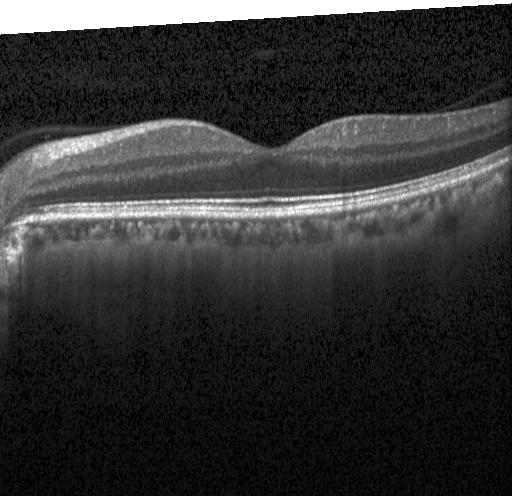

Acquired on a Heidelberg Spectralis, OCT B-scan — The scan shows no evidence of choroidal neovascularization, diabetic macular edema, or drusen.